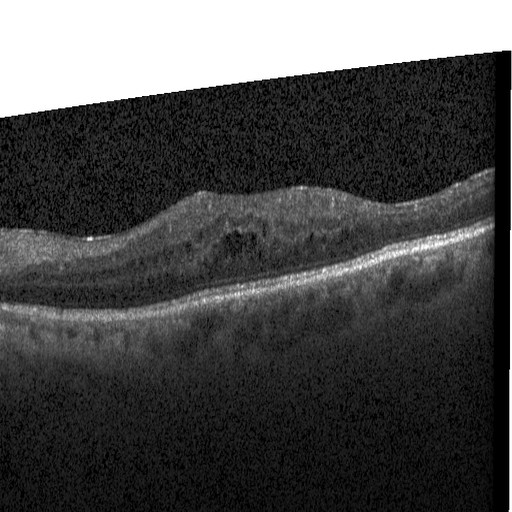

OCT B-scan showing diabetic macular edema.